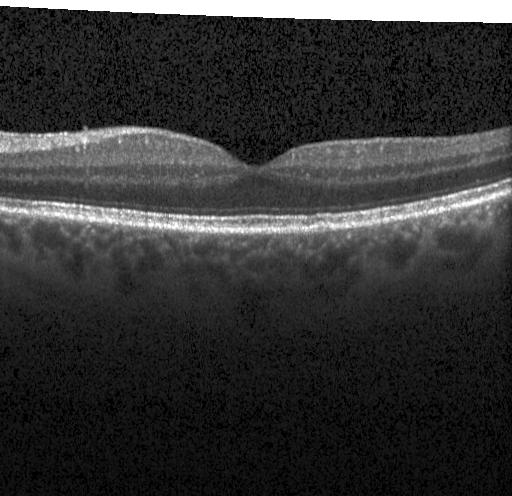

This B-scan demonstrates no evidence of choroidal neovascularization, diabetic macular edema, or drusen.